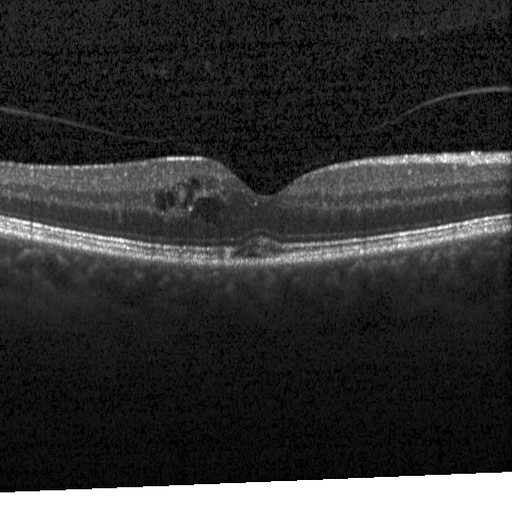

OCT scan showing diabetic macular edema.